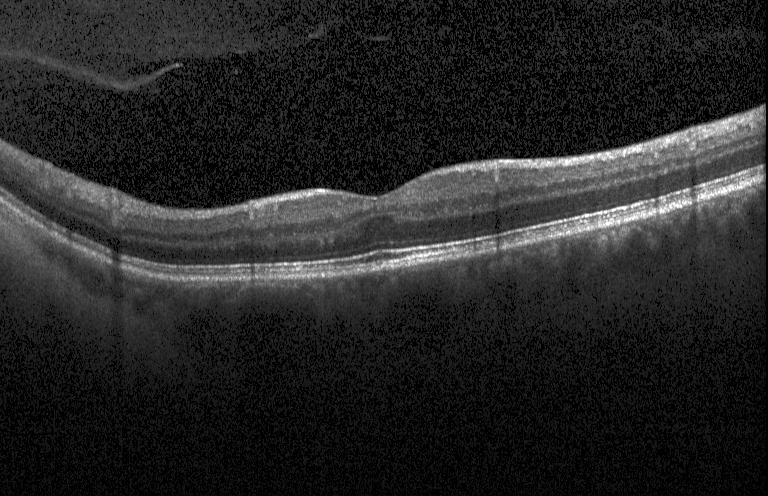
Retinal OCT B-scan. Finding: no choroidal neovascularization, diabetic macular edema, or drusen.